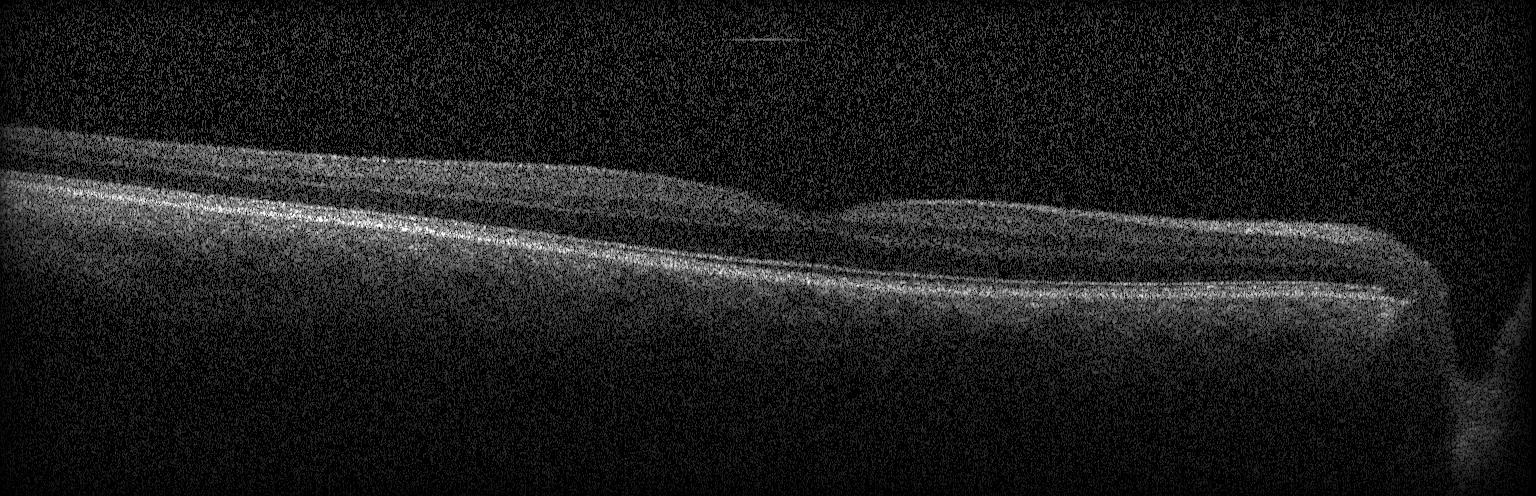

Diagnosis: neither choroidal neovascularization, diabetic macular edema, nor drusen.